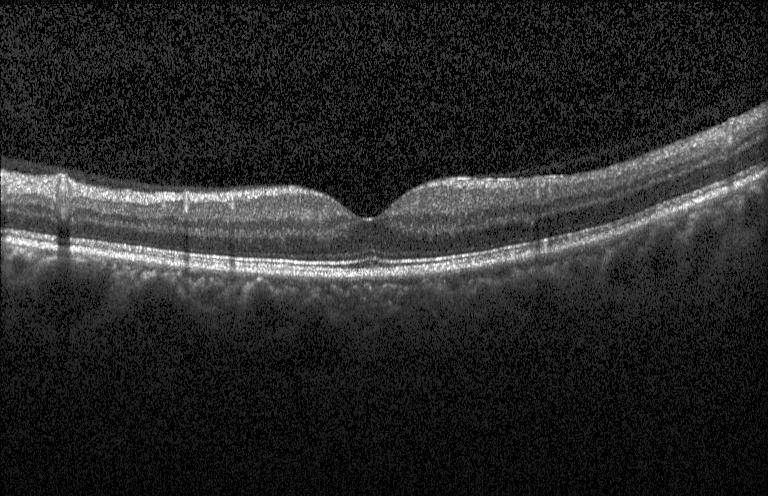 OCT B-scan; SD-OCT
This B-scan demonstrates neither choroidal neovascularization, diabetic macular edema, nor drusen.